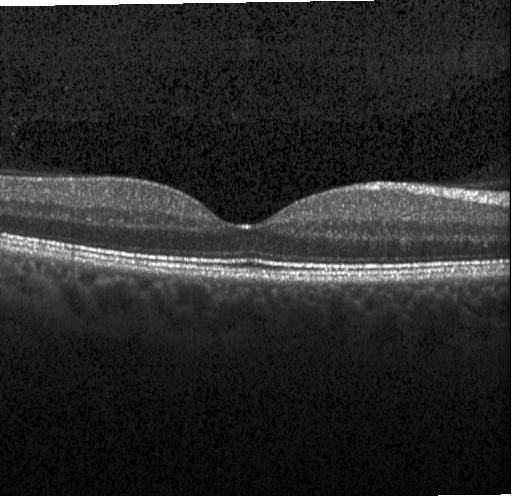 Macular scan. OCT B-scan. Spectral-domain optical coherence tomography — No evidence of choroidal neovascularization, diabetic macular edema, or drusen.